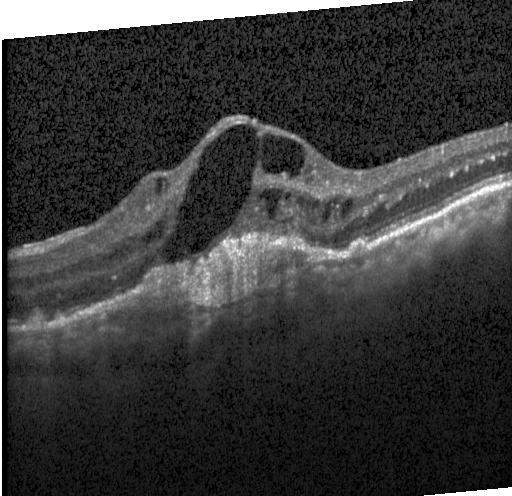

Acquired on a Heidelberg Spectralis, optical coherence tomography scan
Assessment: a choroidal neovascular membrane.